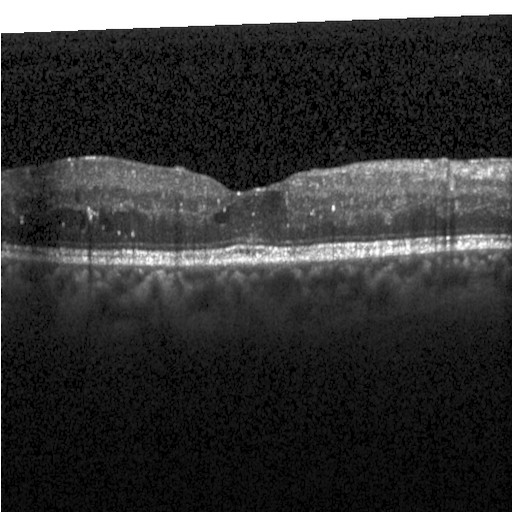
Retinal OCT B-scan.
This B-scan demonstrates diabetic macular edema.